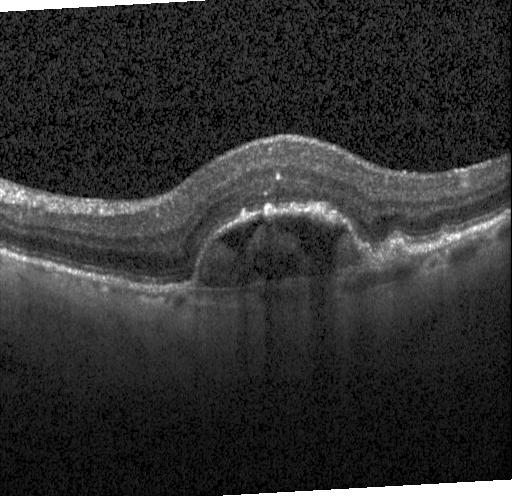
Impression: a choroidal neovascular membrane.